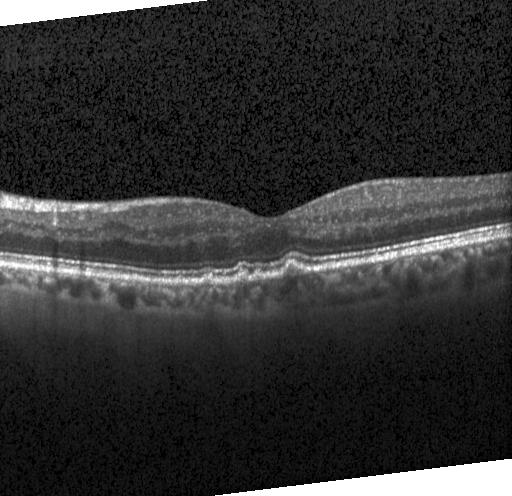 SD-OCT · through the macula · OCT line scan. The scan shows sub-RPE drusenoid deposits.